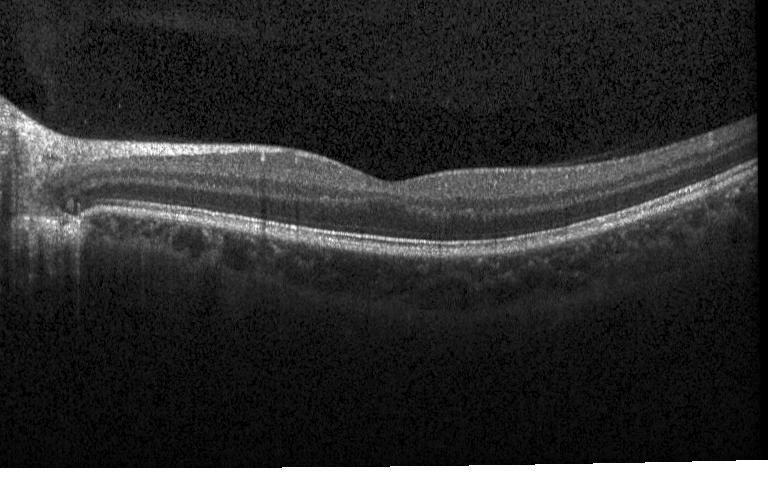

The scan shows no choroidal neovascularization, diabetic macular edema, or drusen.